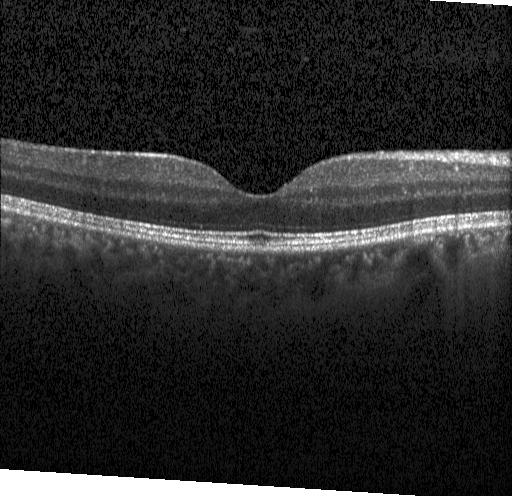 OCT B-scan
Dx: neither CNV, DME, nor drusen.